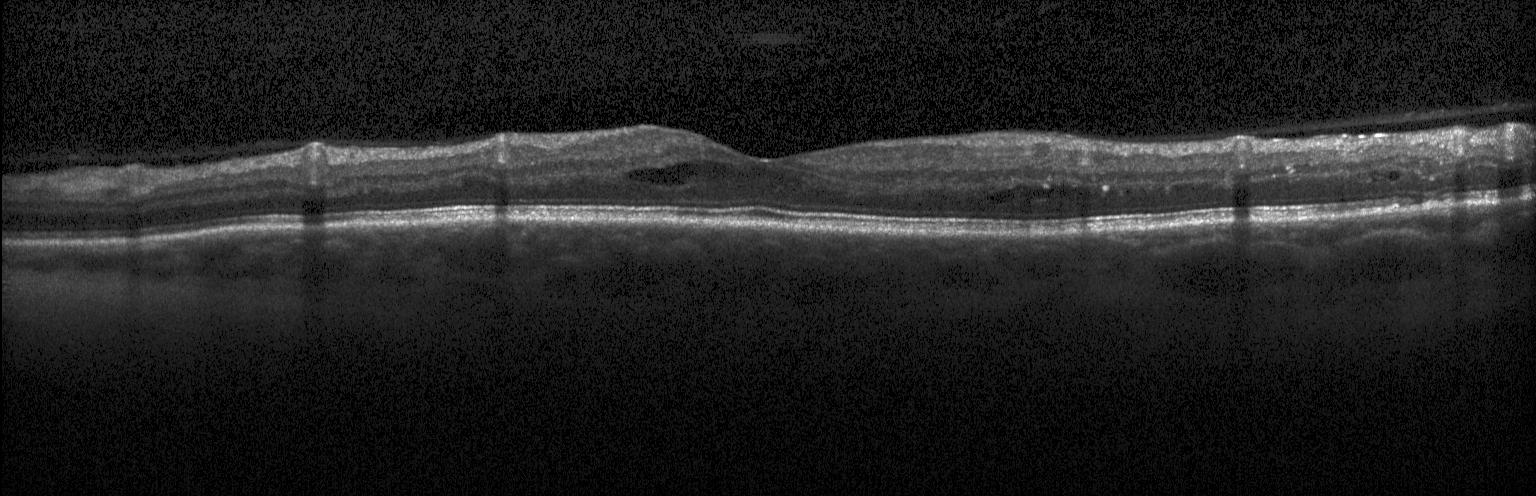

Acquired on a Heidelberg Spectralis; optical coherence tomography B-scan. Impression: diabetic macular edema (DME).